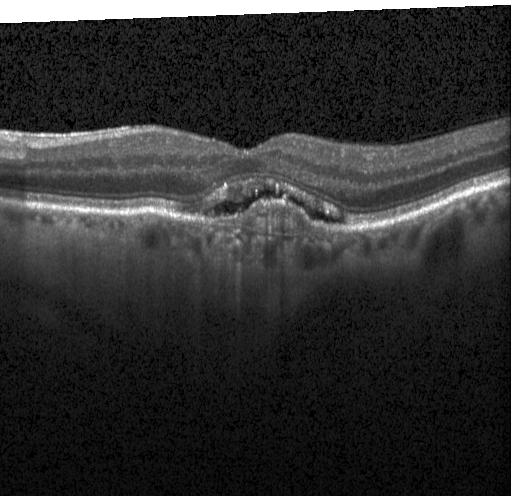

Retinal OCT cross-section, SD-OCT.
Diagnosis: choroidal neovascularization (CNV).